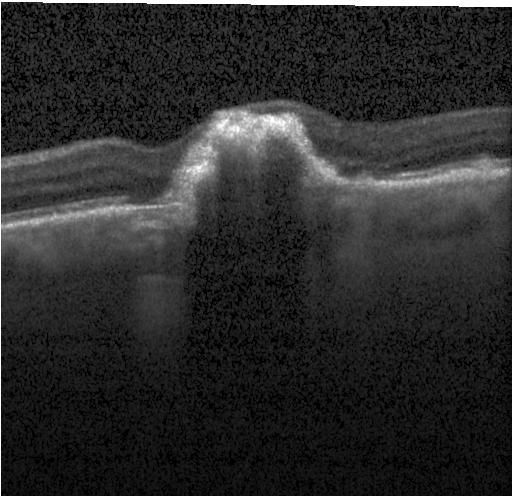 Spectral-domain optical coherence tomography · OCT line scan · centered on the fovea · instrument: Heidelberg Spectralis. The scan shows a choroidal neovascular membrane.